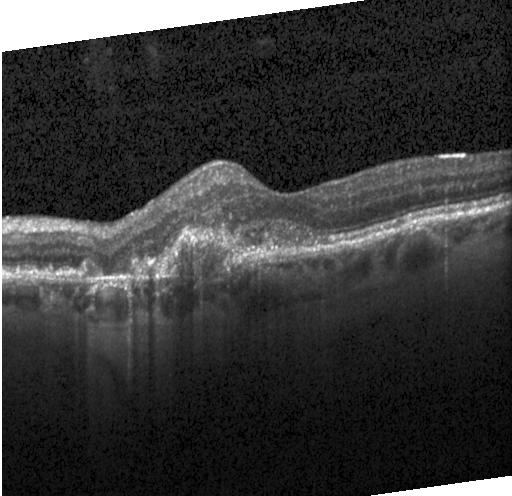

Retinal OCT cross-section · centered on the fovea · instrument: Heidelberg Spectralis
Finding: a choroidal neovascular membrane.